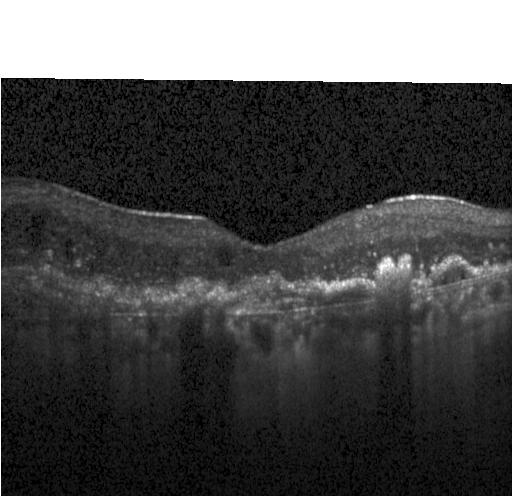 Assessment: choroidal neovascularization.